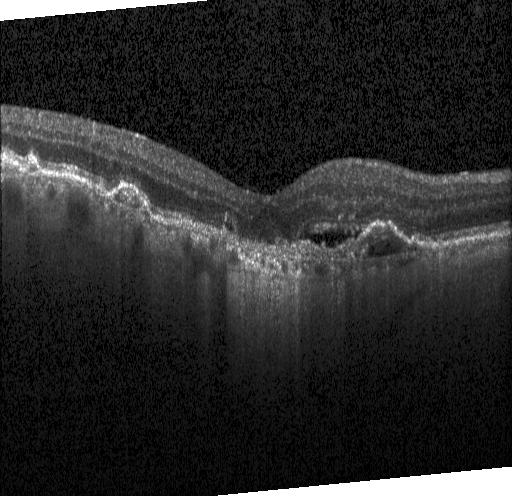 Retinal OCT B-scan. Acquired on a Heidelberg Spectralis. This B-scan demonstrates a choroidal neovascular membrane.